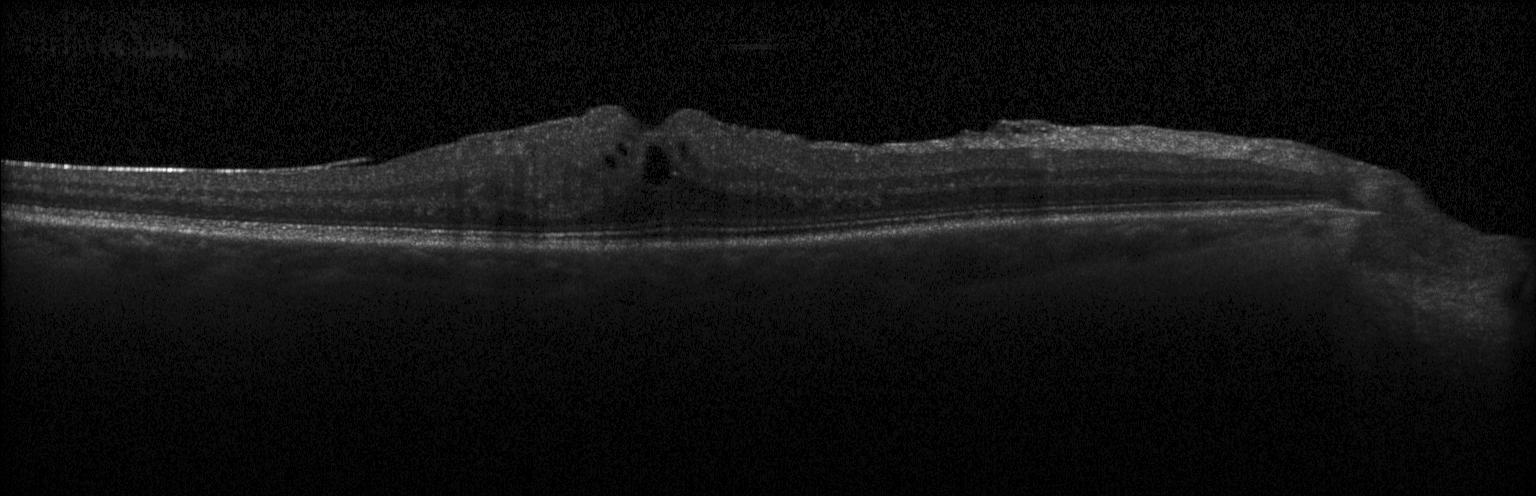
OCT B-scan showing diabetic macular edema.